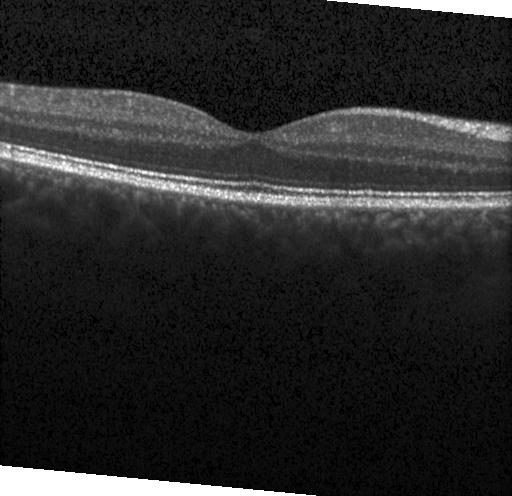
The scan shows no evidence of choroidal neovascularization, diabetic macular edema, or drusen.